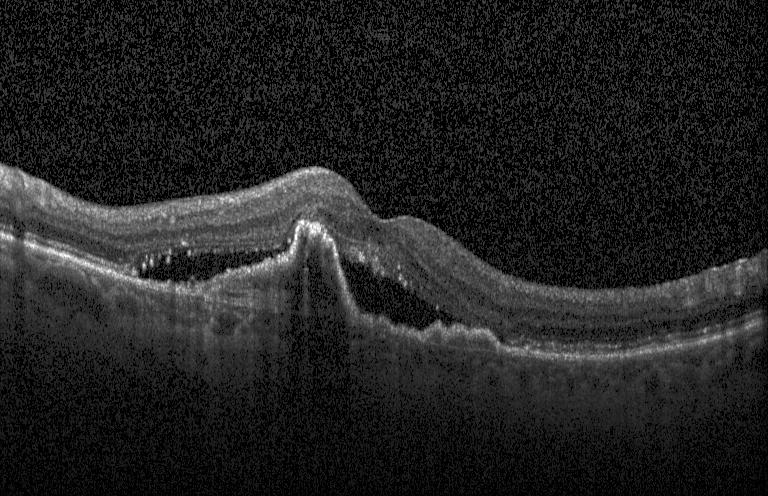

A choroidal neovascular membrane.